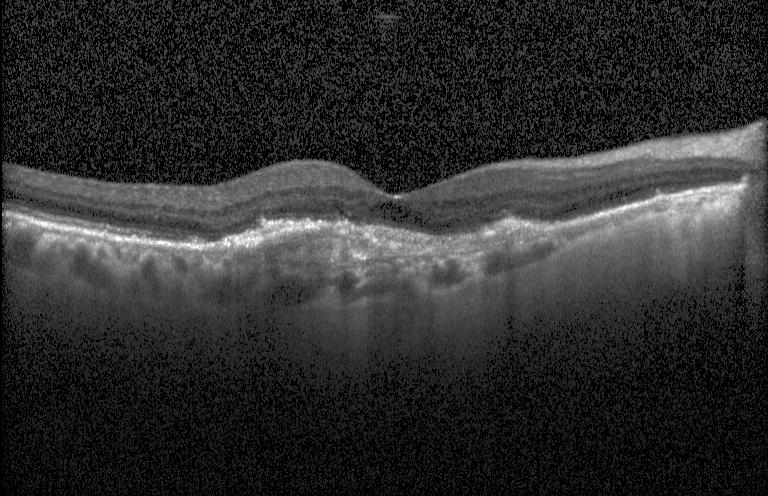 Retinal OCT cross-section. A choroidal neovascular membrane.